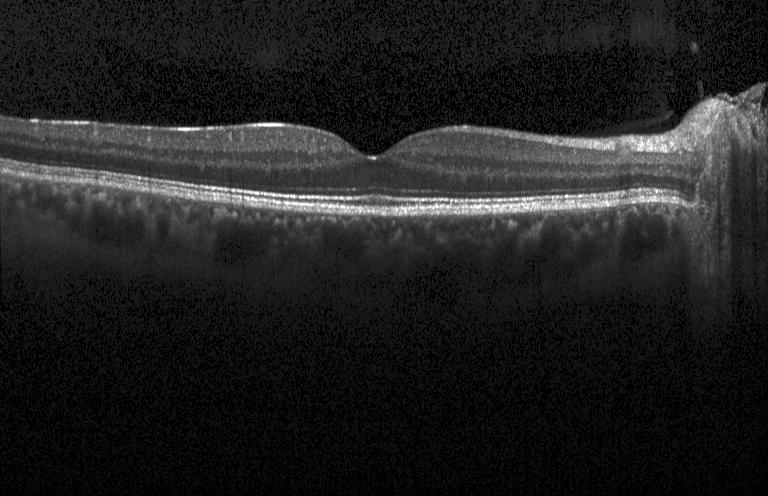
OCT B-scan.
Assessment: no evidence of CNV, DME, or drusen.